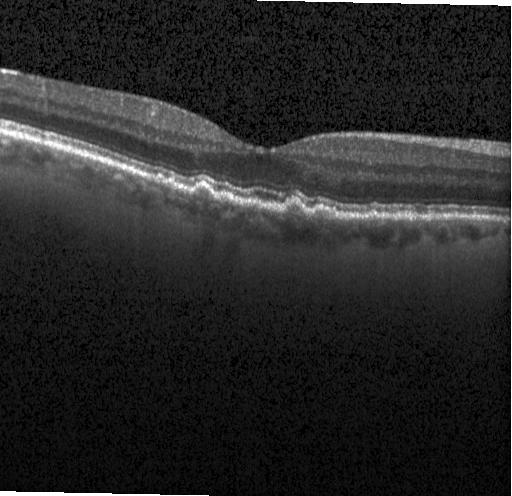 Dx: sub-RPE drusenoid deposits.